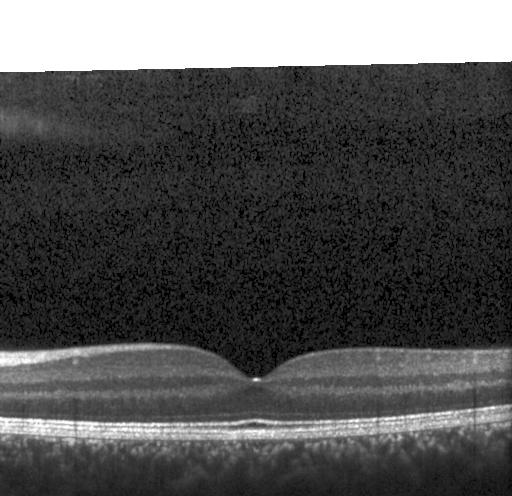

Spectral-domain OCT B-scan: no CNV, DME, or drusen.